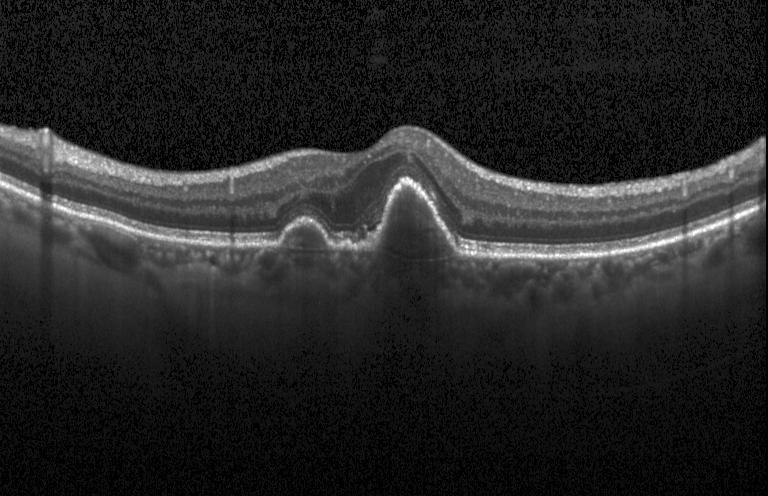 Spectral-domain optical coherence tomography, retinal OCT B-scan, centered on the fovea. This B-scan demonstrates a choroidal neovascular membrane.